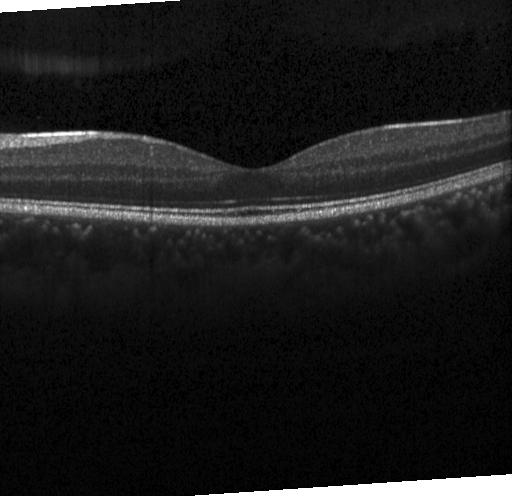

Acquired on a Heidelberg Spectralis; retinal OCT cross-section; horizontal scan through the fovea. Finding: no choroidal neovascularization, no diabetic macular edema, and no drusen.